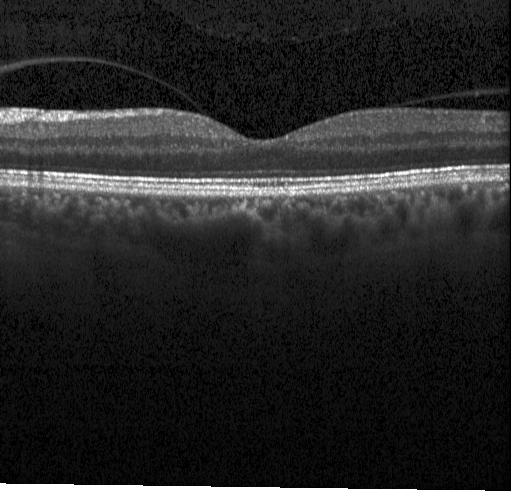

Finding: no evidence of CNV, DME, or drusen.